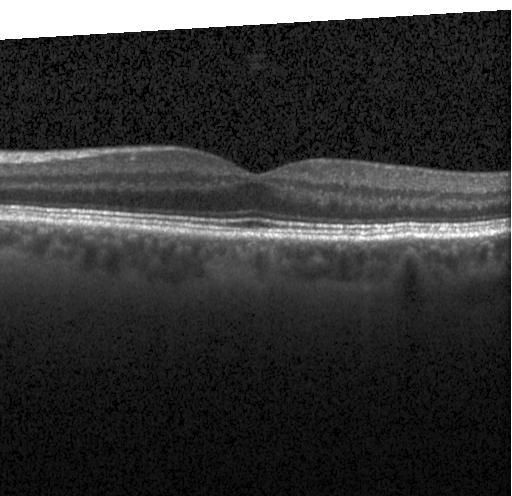
Spectral-domain optical coherence tomography, retinal OCT B-scan, acquired on a Heidelberg Spectralis.
Dx: no evidence of CNV, DME, or drusen.